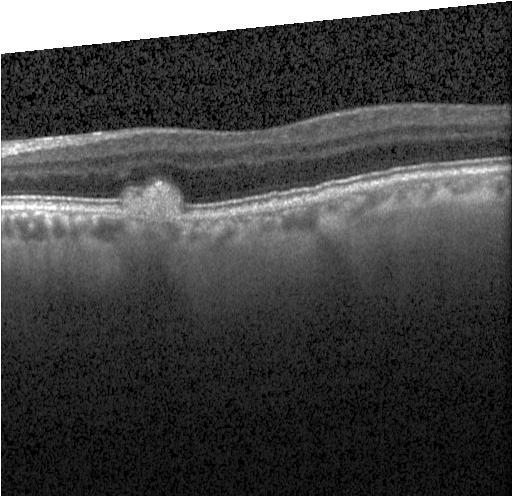

OCT B-scan; acquired on a Heidelberg Spectralis. OCT finding: a choroidal neovascular membrane.